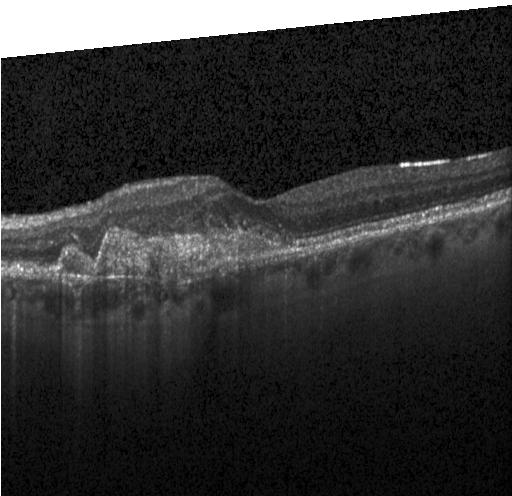 Diagnosis: CNV.